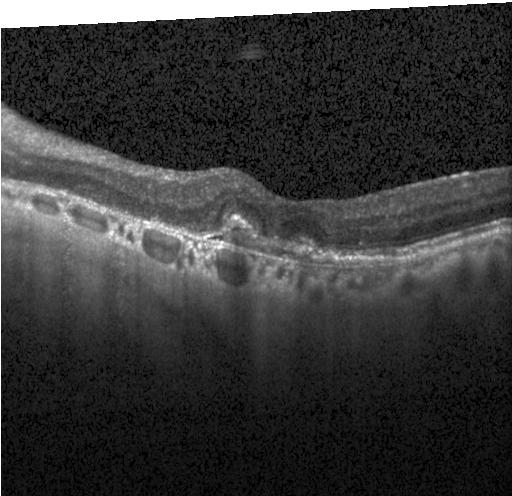

OCT finding: CNV.